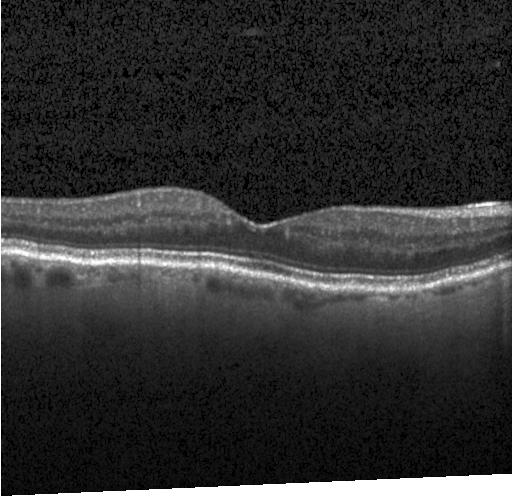

Macular OCT: neither CNV, DME, nor drusen.